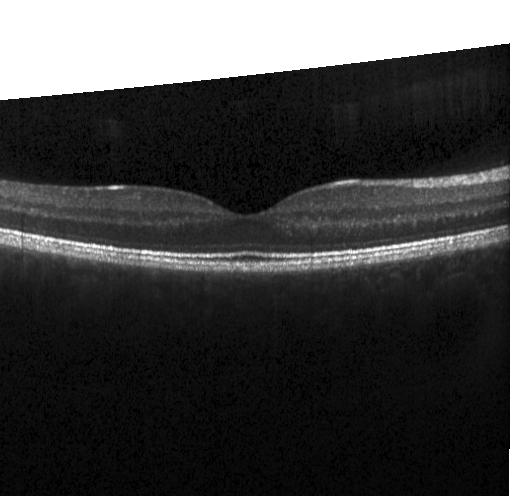 Acquired on a Heidelberg Spectralis. Spectral-domain optical coherence tomography. Optical coherence tomography scan — OCT finding: neither choroidal neovascularization, diabetic macular edema, nor drusen.